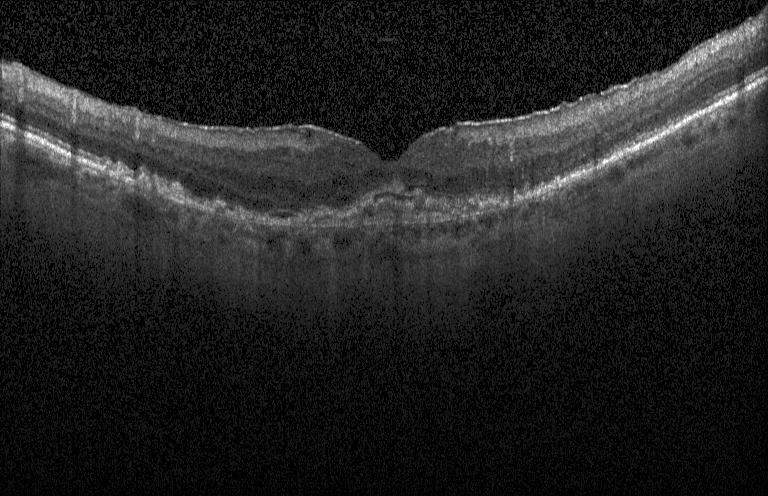

OCT B-scan. Impression: CNV.